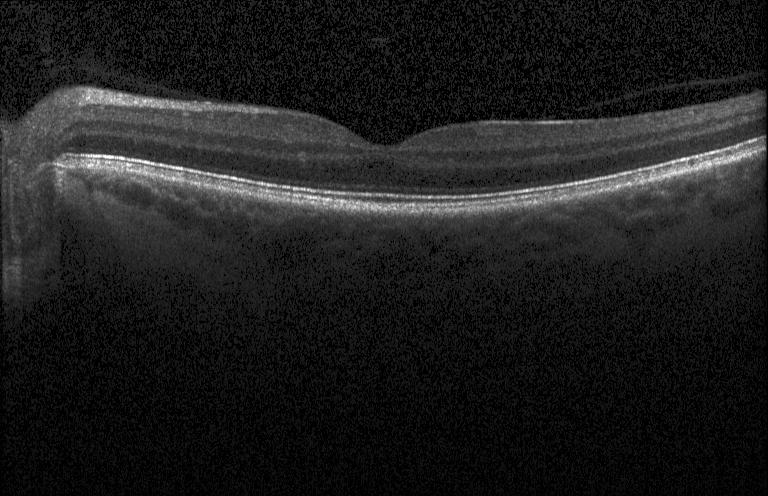

OCT B-scan.
Impression: neither choroidal neovascularization, diabetic macular edema, nor drusen.